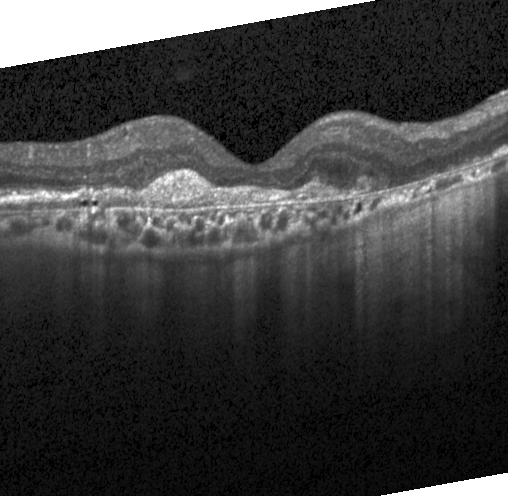

Spectral-domain optical coherence tomography; optical coherence tomography B-scan. Diagnosis: a choroidal neovascular membrane.